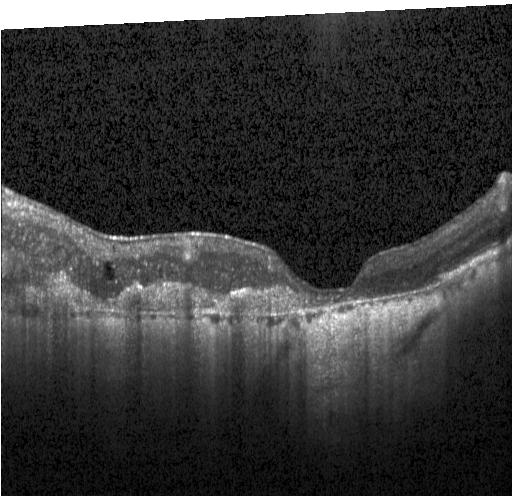 Macular scan, retinal OCT B-scan, instrument: Heidelberg Spectralis. Finding: a choroidal neovascular membrane.